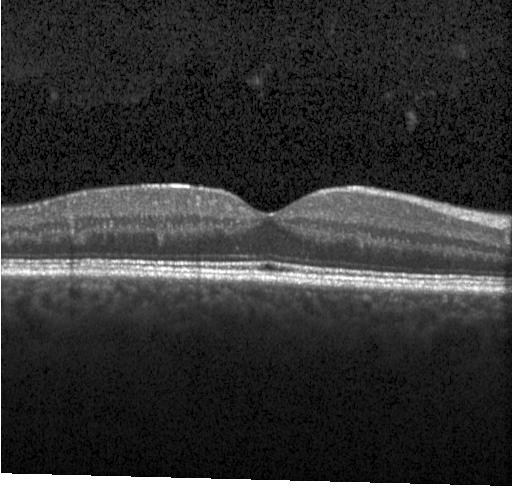
Heidelberg Spectralis OCT system. Retinal OCT cross-section. Spectral-domain OCT — OCT finding: no choroidal neovascularization, diabetic macular edema, or drusen.